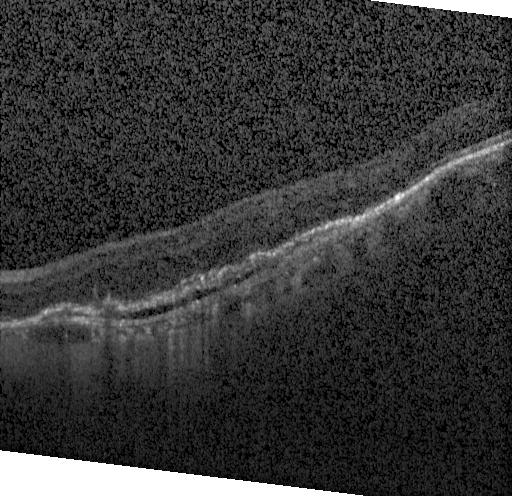
OCT line scan
OCT finding: choroidal neovascularization.